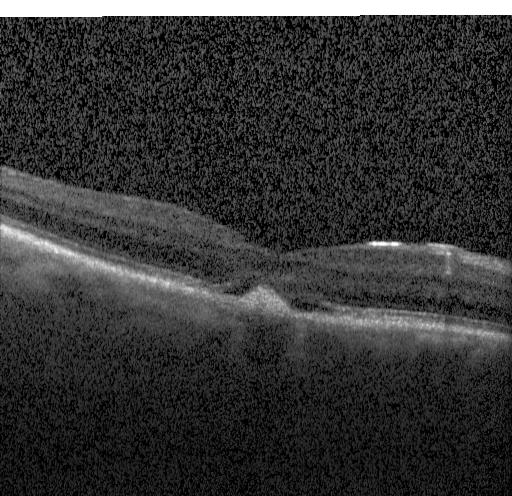
OCT scan showing a choroidal neovascular membrane.